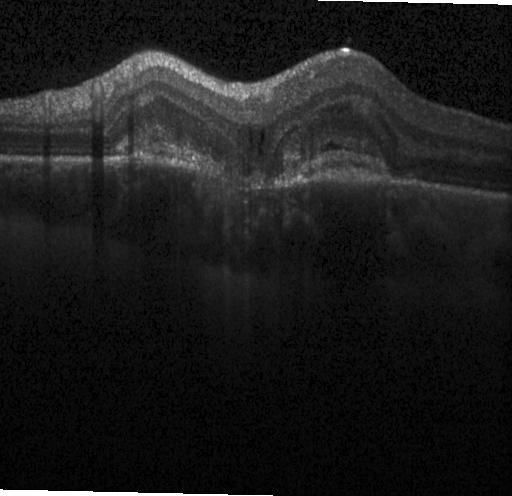
OCT finding: a choroidal neovascular membrane.